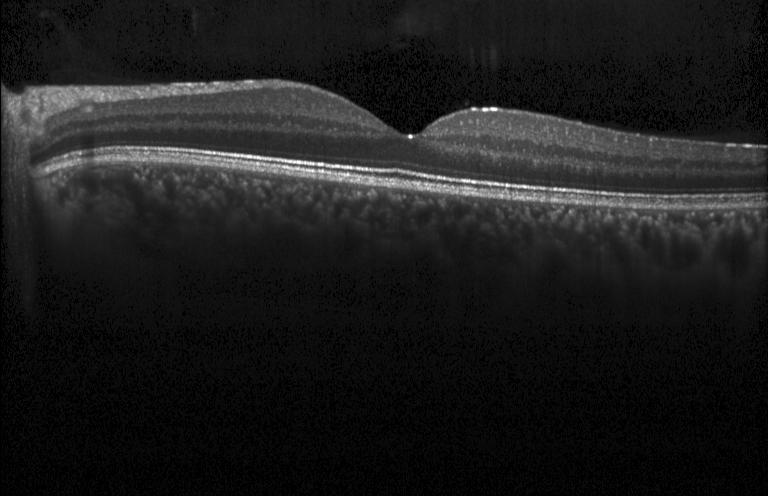 This B-scan demonstrates neither choroidal neovascularization, diabetic macular edema, nor drusen.